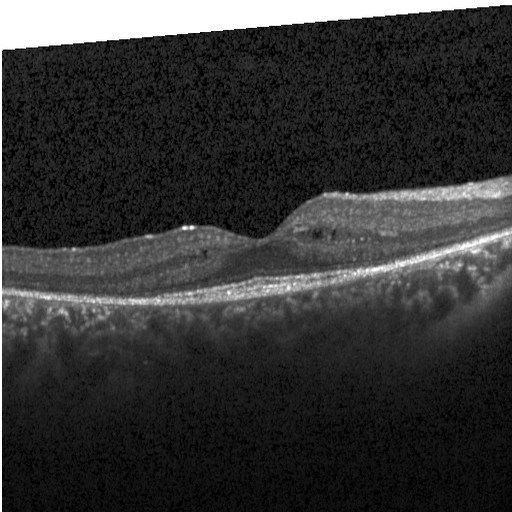

Assessment: diabetic macular edema.